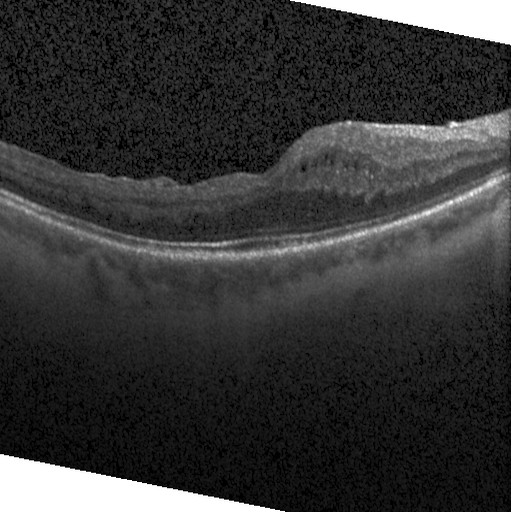
Spectral-domain OCT B-scan: DME.